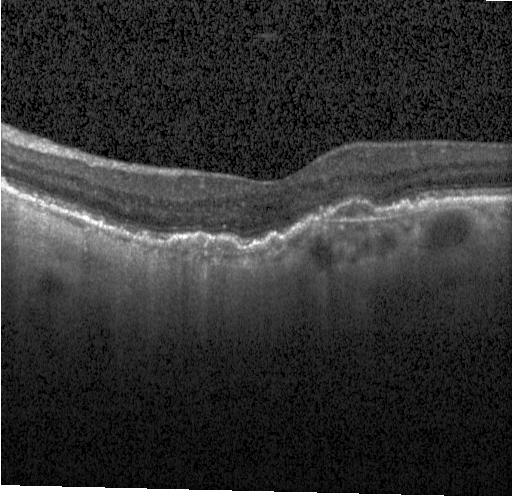
Optical coherence tomography B-scan; SD-OCT.
The scan shows CNV.